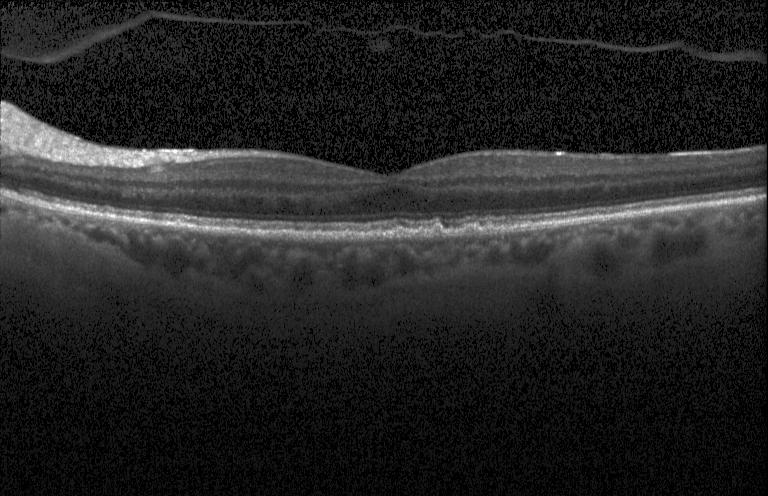
Assessment: multiple drusen.